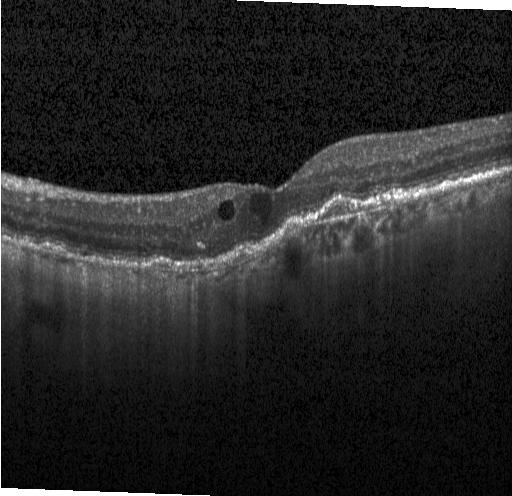
OCT B-scan.
This B-scan demonstrates a choroidal neovascular membrane.